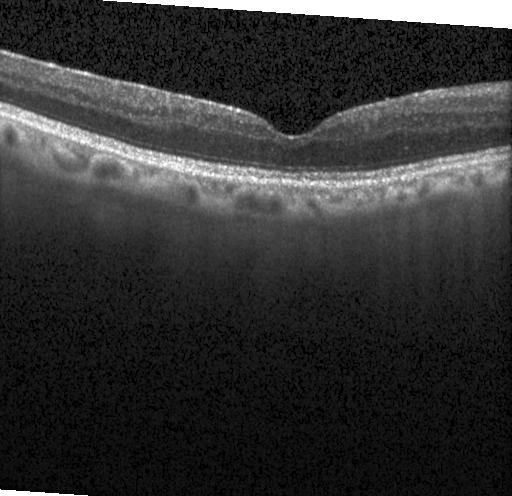

Macular OCT: no choroidal neovascularization, diabetic macular edema, or drusen.